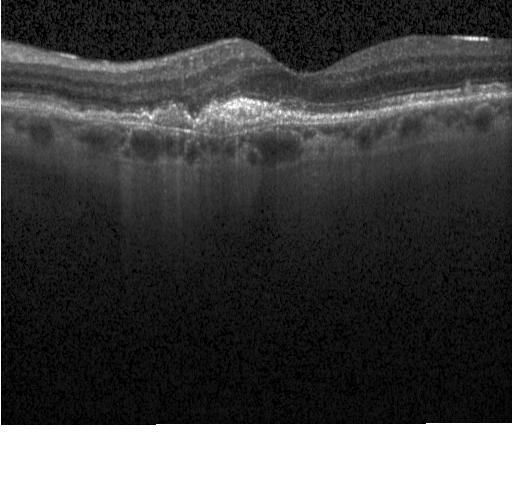 OCT B-scan.
A choroidal neovascular membrane.